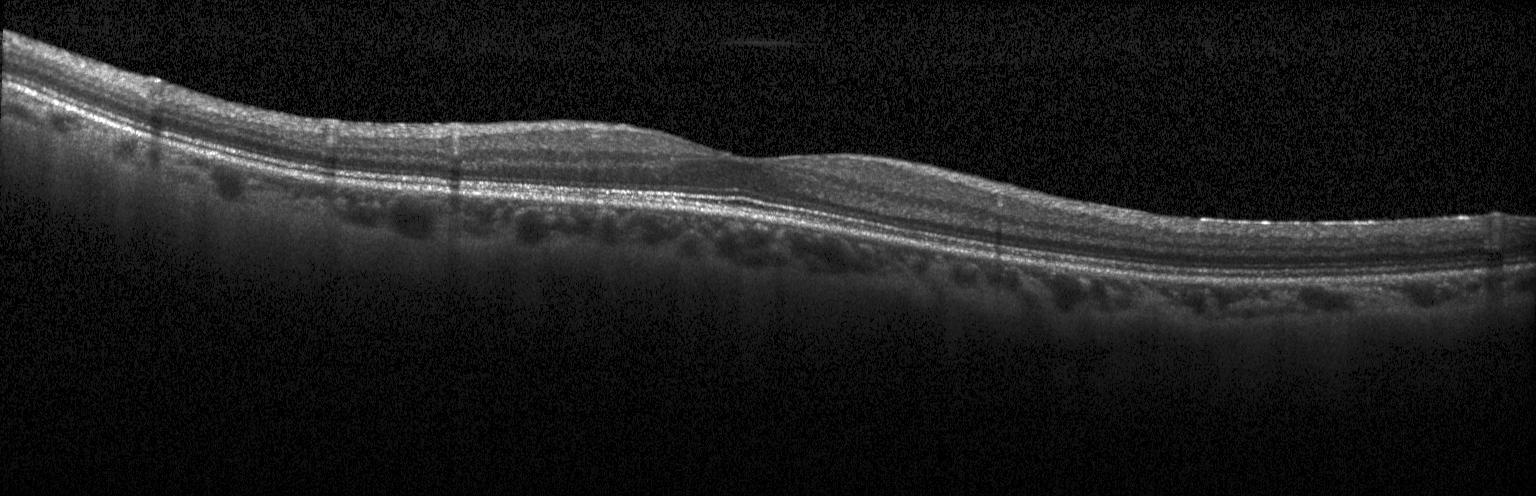
Spectral-domain optical coherence tomography, retinal OCT B-scan.
Assessment: no evidence of choroidal neovascularization, diabetic macular edema, or drusen.